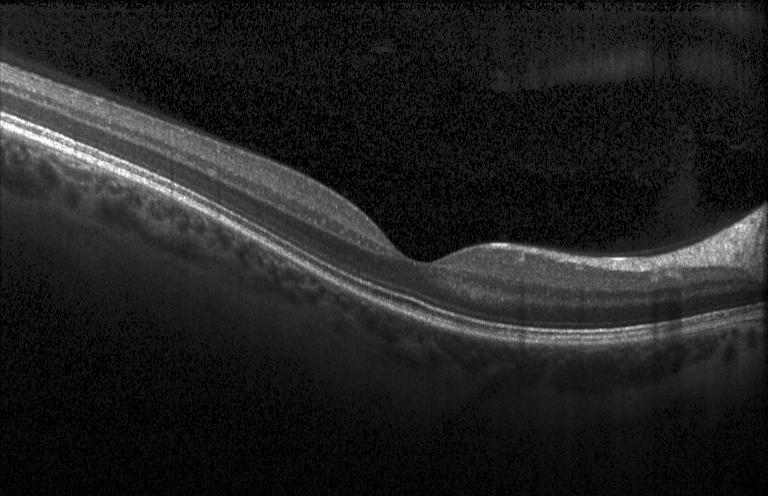 Instrument: Heidelberg Spectralis, spectral-domain OCT, retinal OCT cross-section, horizontal scan through the fovea — Impression: neither choroidal neovascularization, diabetic macular edema, nor drusen.